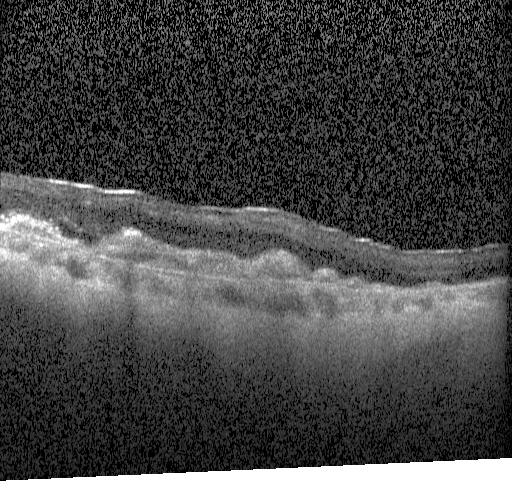

SD-OCT, acquired on a Heidelberg Spectralis, retinal OCT cross-section, horizontal scan through the fovea — Diagnosis: a choroidal neovascular membrane.